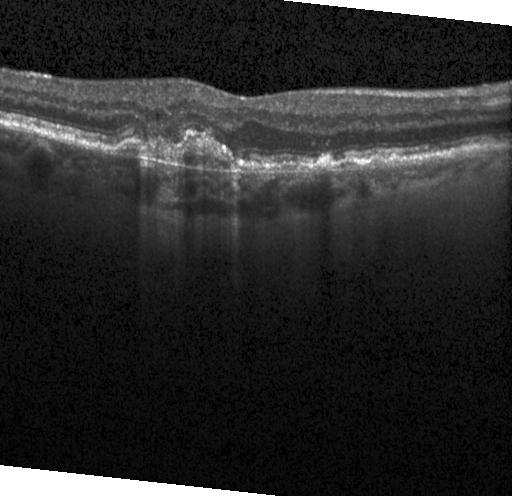 Finding: CNV.